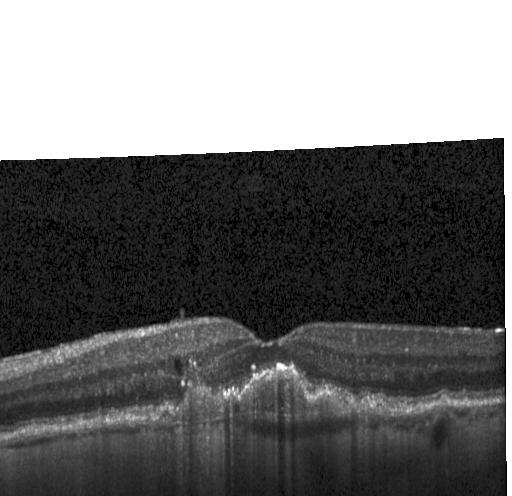
Macular OCT demonstrating choroidal neovascularization.